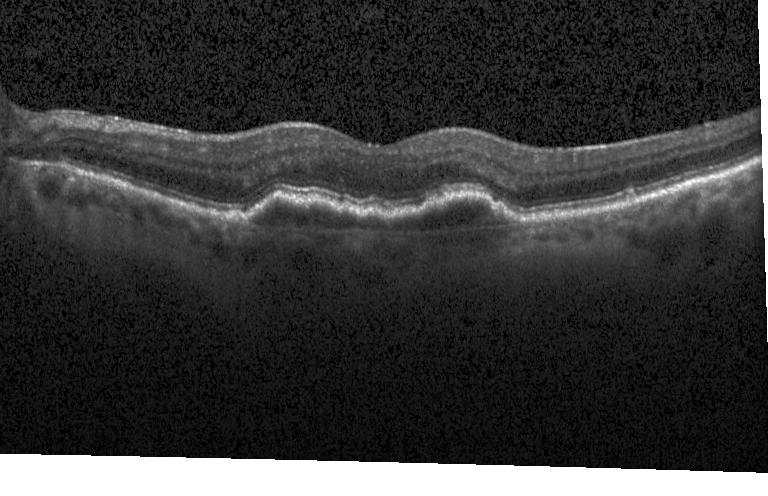
Fovea-centered; optical coherence tomography scan; SD-OCT — Impression: CNV.